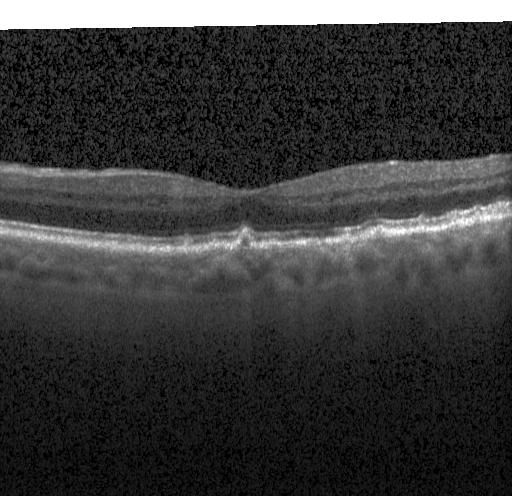

Diagnosis: drusen.